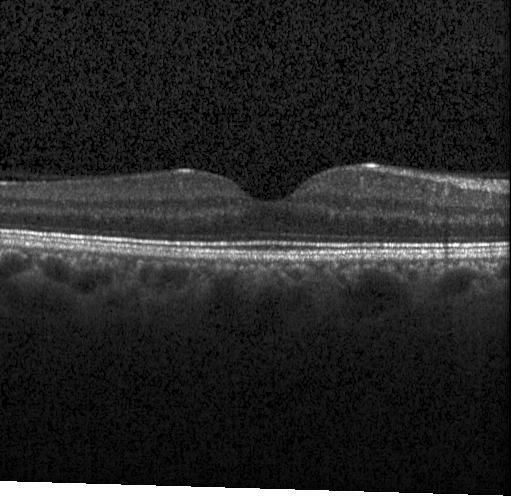 Finding: no choroidal neovascularization, no diabetic macular edema, and no drusen.